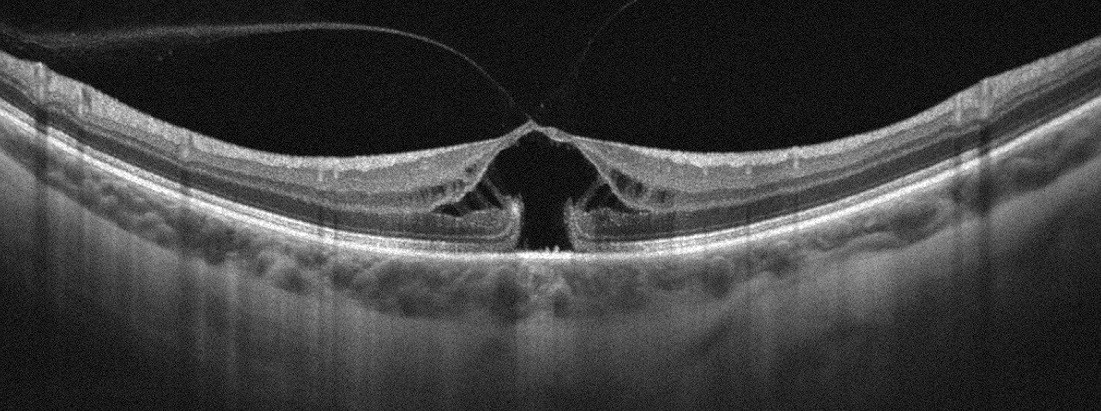
Retinal OCT cross-section, through the macula, Optovue Avanti RTVue XR — Dx: VID.